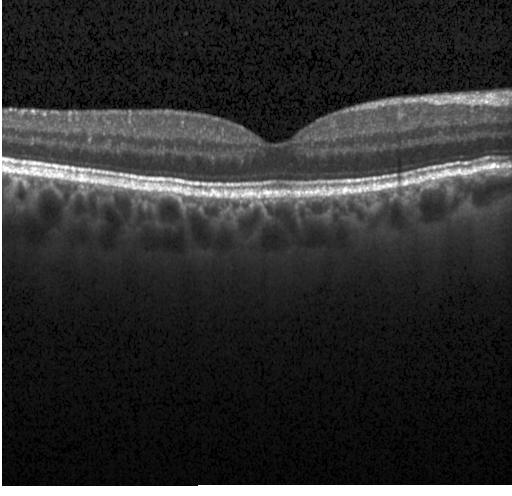
Centered on the fovea; retinal OCT B-scan.
Impression: neither choroidal neovascularization, diabetic macular edema, nor drusen.